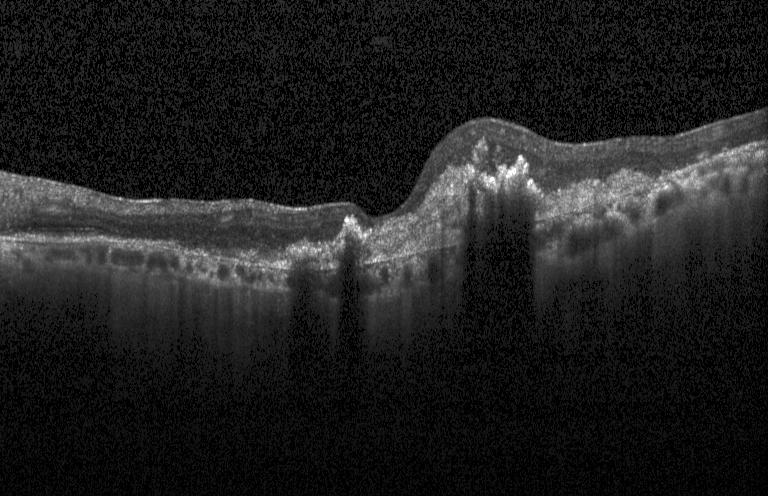
Macular OCT: a choroidal neovascular membrane.